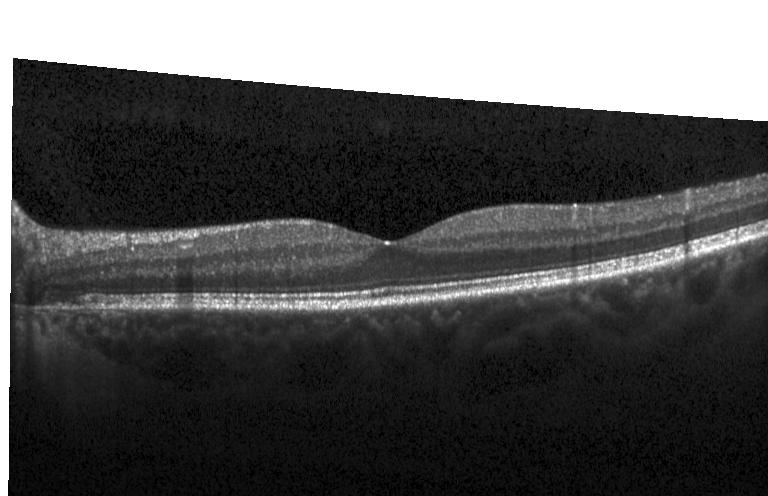

OCT line scan.
Macular OCT: no evidence of CNV, DME, or drusen.